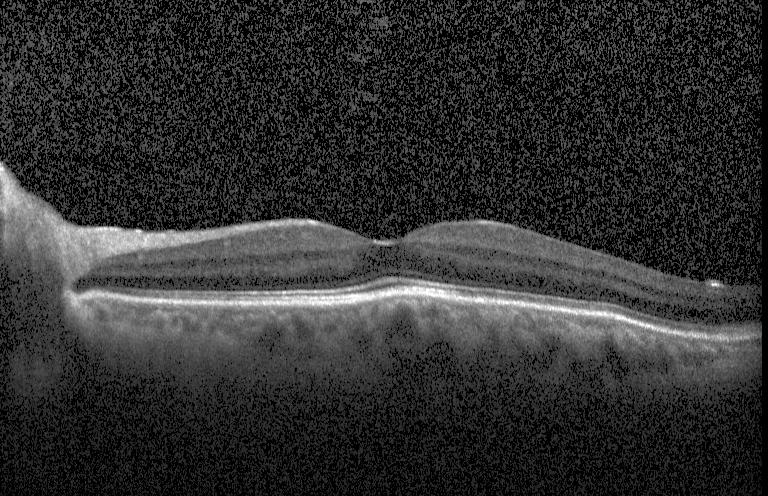

Spectral-domain optical coherence tomography; optical coherence tomography scan; instrument: Heidelberg Spectralis.
Impression: no evidence of choroidal neovascularization, diabetic macular edema, or drusen.